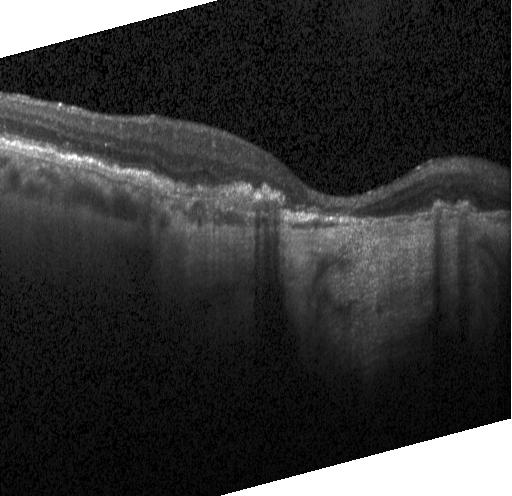
Impression: choroidal neovascularization.